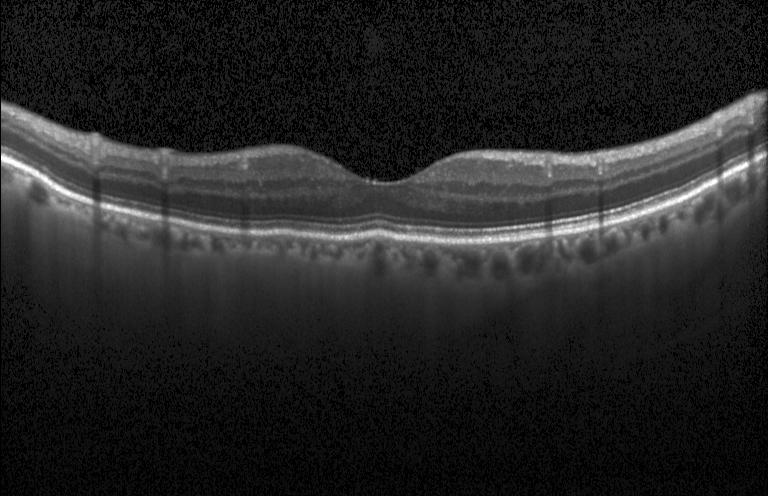

Finding: no CNV, no DME, and no drusen.